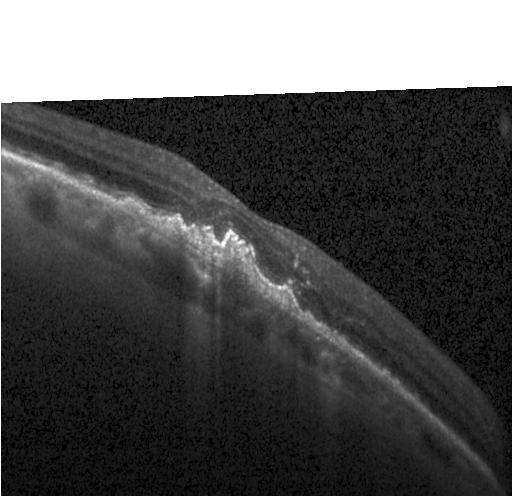
Spectral-domain OCT, Heidelberg Spectralis OCT system, optical coherence tomography B-scan, through the macula — Impression: choroidal neovascularization.